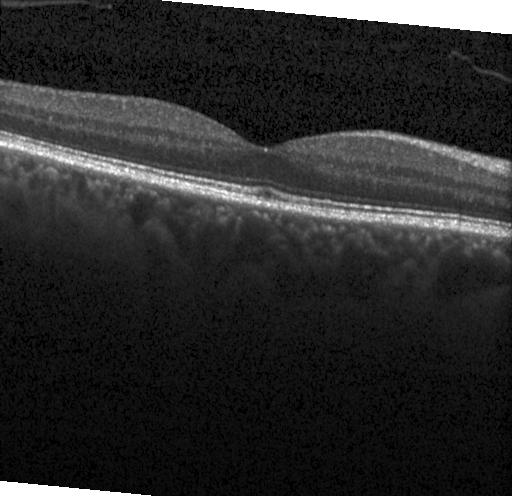 Assessment: no choroidal neovascularization, diabetic macular edema, or drusen.